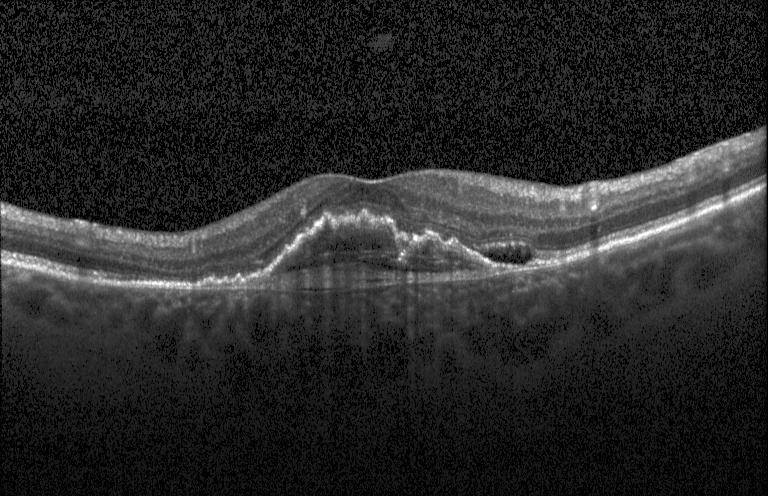 Optical coherence tomography B-scan; Heidelberg Spectralis; spectral-domain optical coherence tomography; horizontal scan through the fovea.
Impression: choroidal neovascularization (CNV).